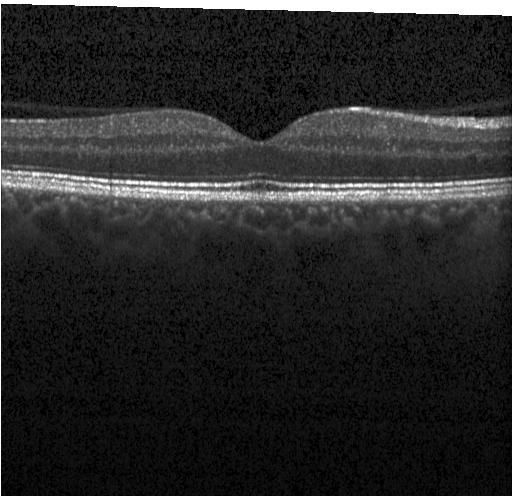

OCT B-scan showing no CNV, DME, or drusen.